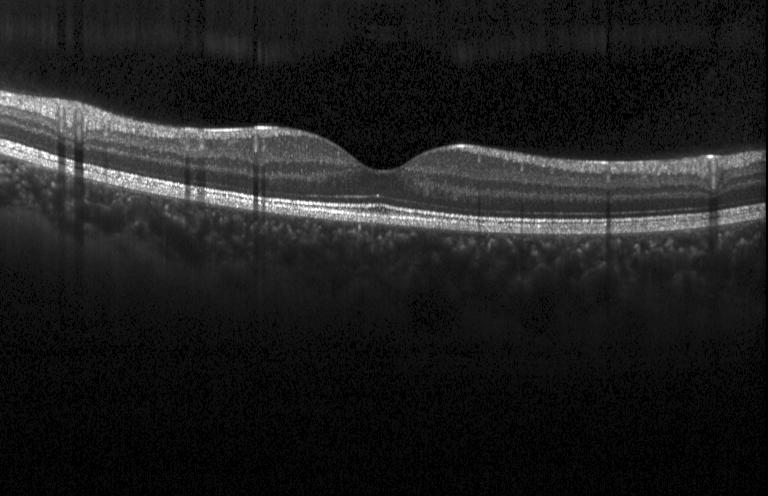

Retinal OCT cross-section, macular scan — Assessment: no CNV, no DME, and no drusen.